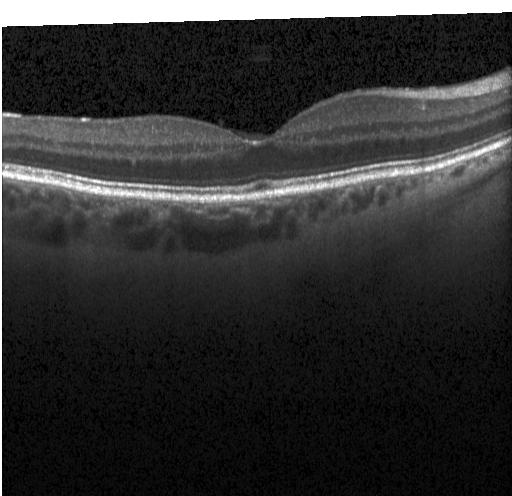

Macular scan. Retinal OCT B-scan. Spectral-domain OCT — Impression: no evidence of choroidal neovascularization, diabetic macular edema, or drusen.